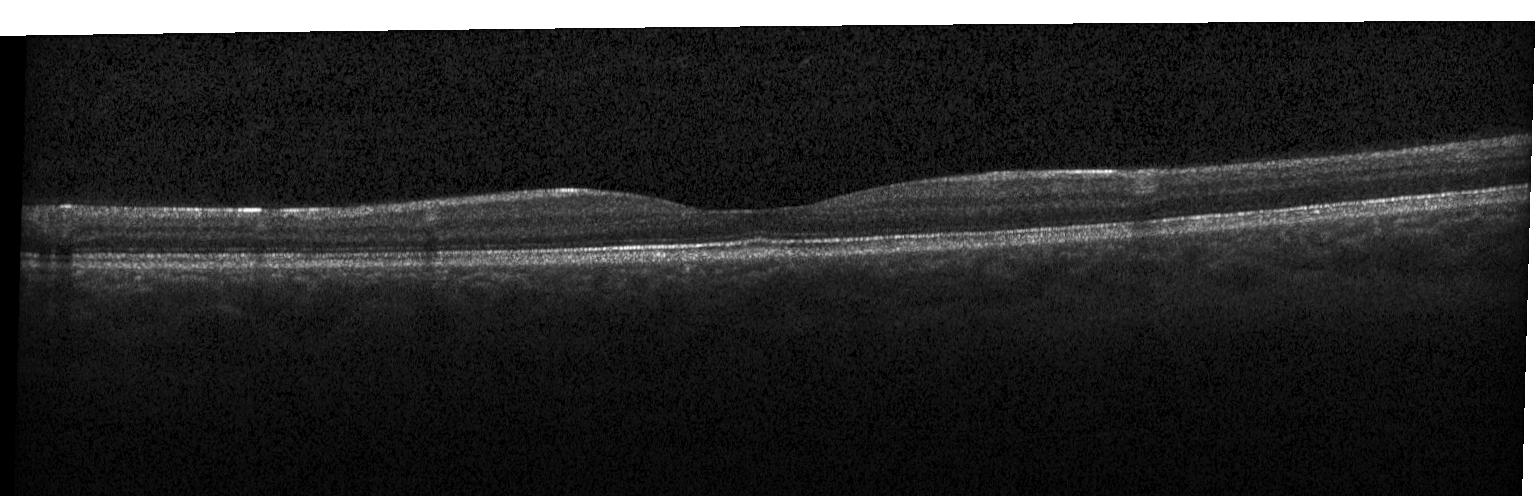
Retinal OCT B-scan. OCT finding: no evidence of choroidal neovascularization, diabetic macular edema, or drusen.